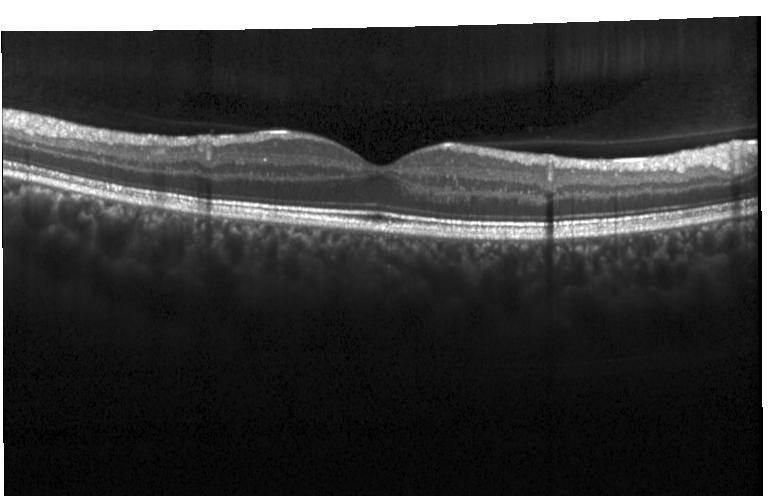

SD-OCT; instrument: Heidelberg Spectralis; retinal OCT cross-section; fovea-centered.
The scan shows no CNV, no DME, and no drusen.